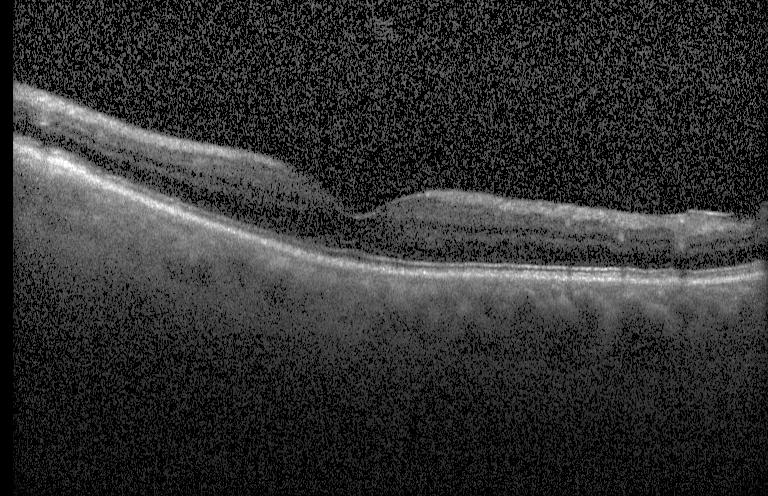 Spectral-domain OCT B-scan: no choroidal neovascularization, diabetic macular edema, or drusen.